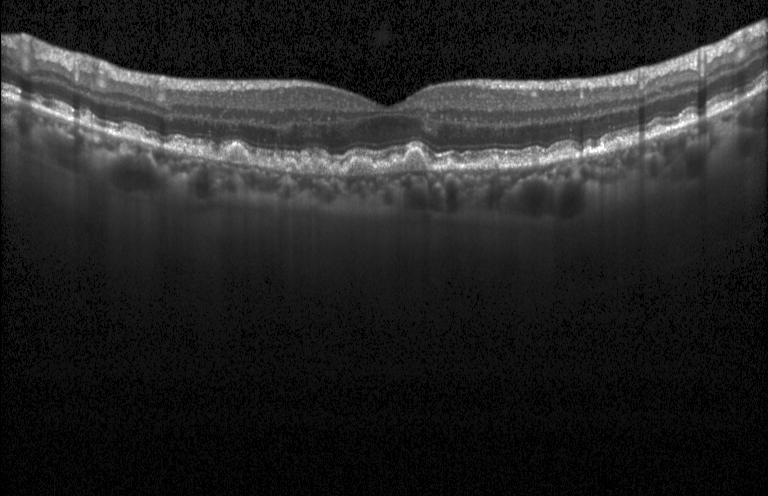 Impression: drusen.